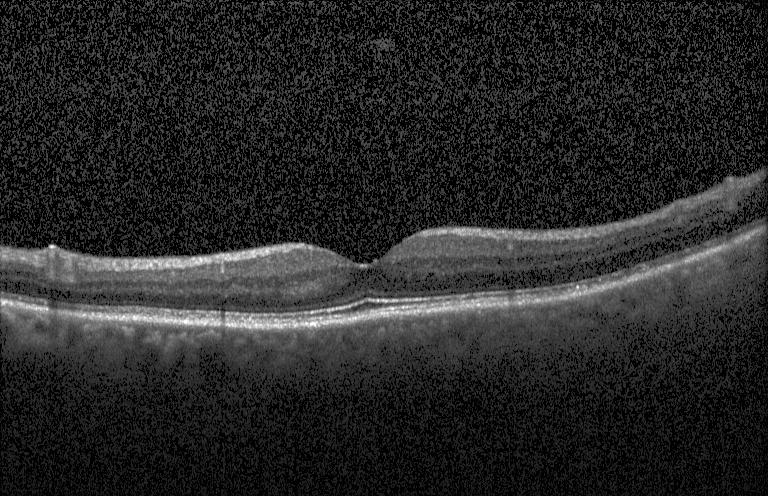 Retinal OCT cross-section
Impression: no CNV, no DME, and no drusen.